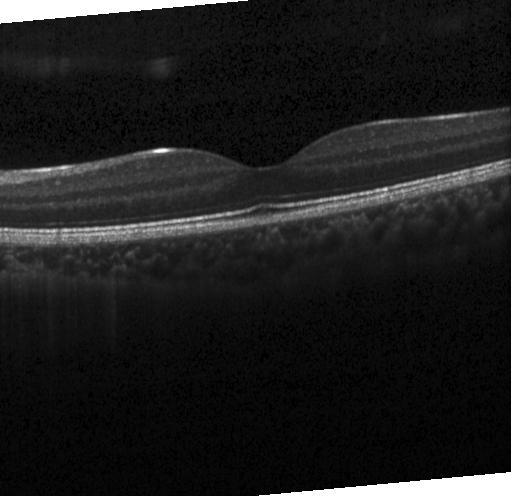
Fovea-centered, retinal OCT B-scan.
The scan shows no CNV, no DME, and no drusen.